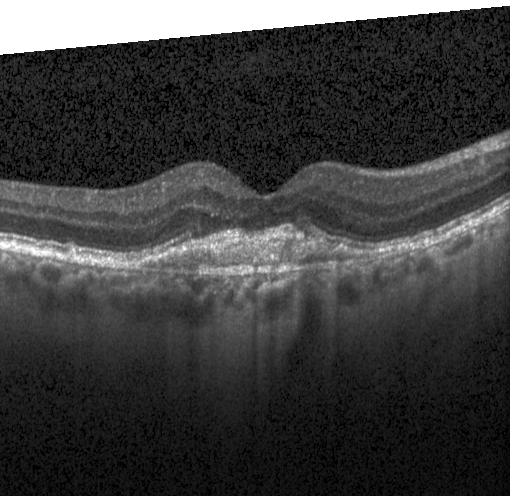 SD-OCT, macular scan, acquired on a Heidelberg Spectralis, retinal OCT B-scan
Impression: choroidal neovascularization (CNV).